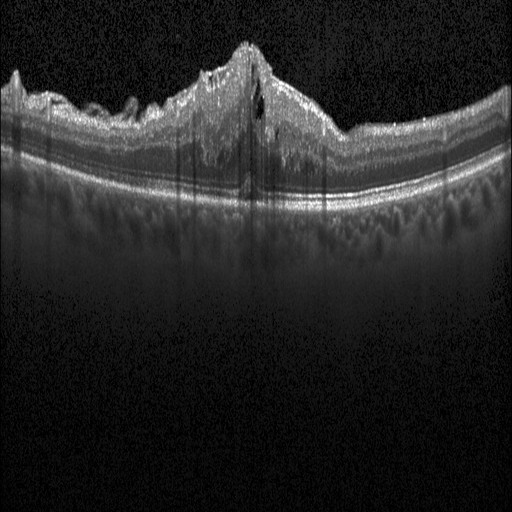

Macular OCT: diabetic macular edema (DME).